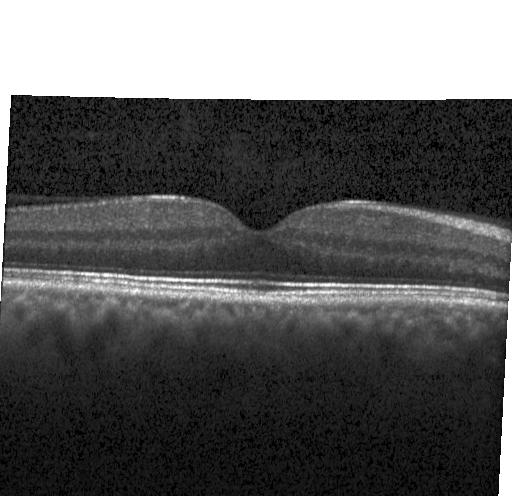
Heidelberg Spectralis; retinal OCT cross-section; through the macula; spectral-domain optical coherence tomography.
Assessment: neither CNV, DME, nor drusen.